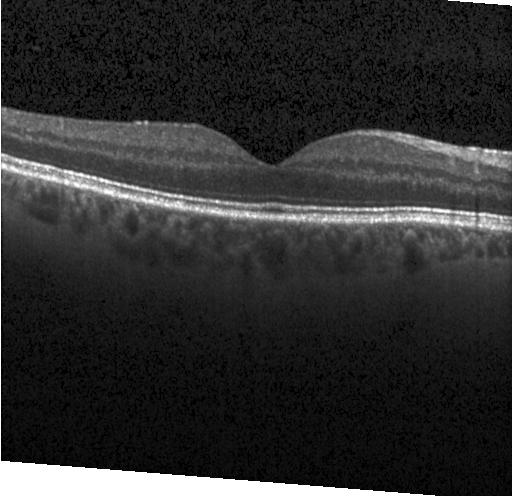
No CNV, DME, or drusen.